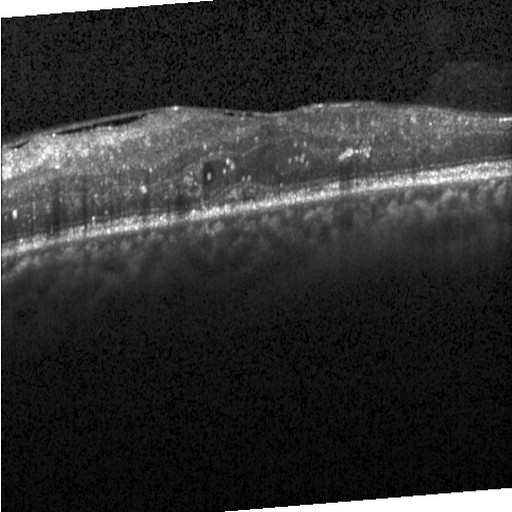 Optical coherence tomography B-scan.
Finding: DME.